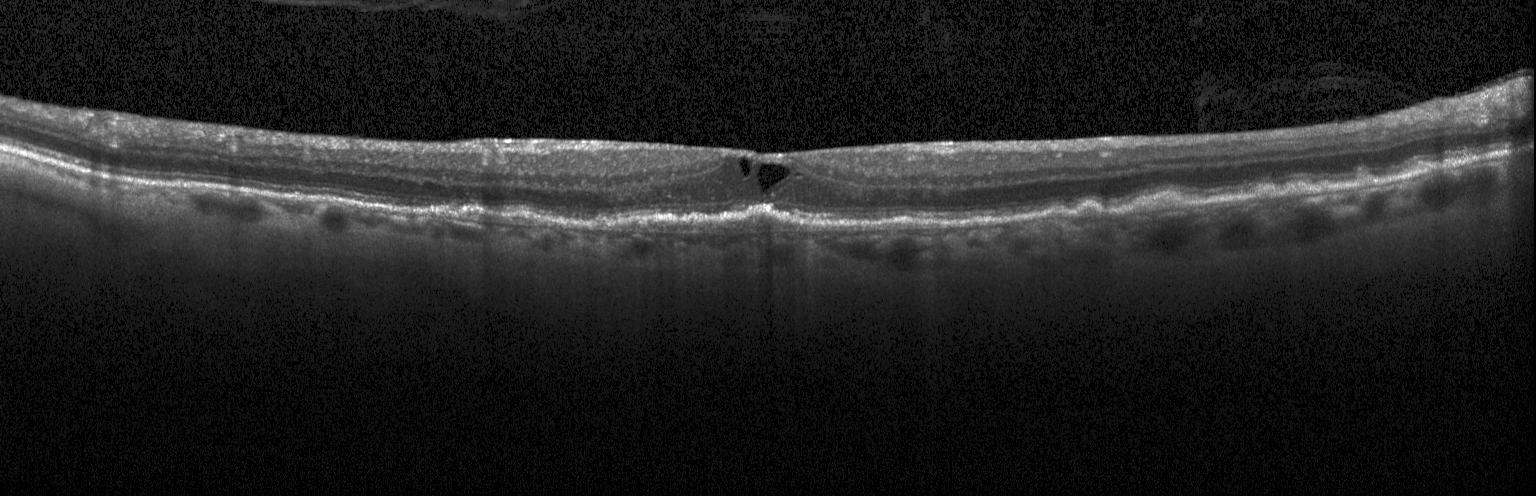

Instrument: Heidelberg Spectralis; OCT B-scan.
Diagnosis: choroidal neovascularization.